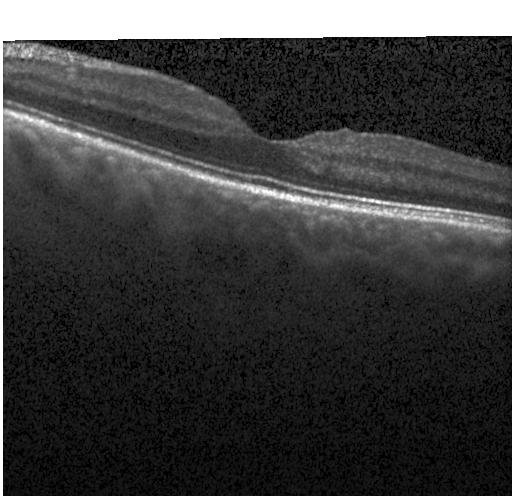

Assessment: no evidence of choroidal neovascularization, diabetic macular edema, or drusen.